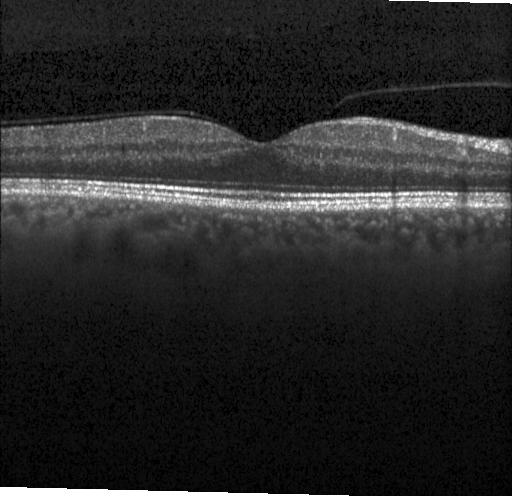
Instrument: Heidelberg Spectralis; retinal OCT cross-section.
Finding: no choroidal neovascularization, no diabetic macular edema, and no drusen.